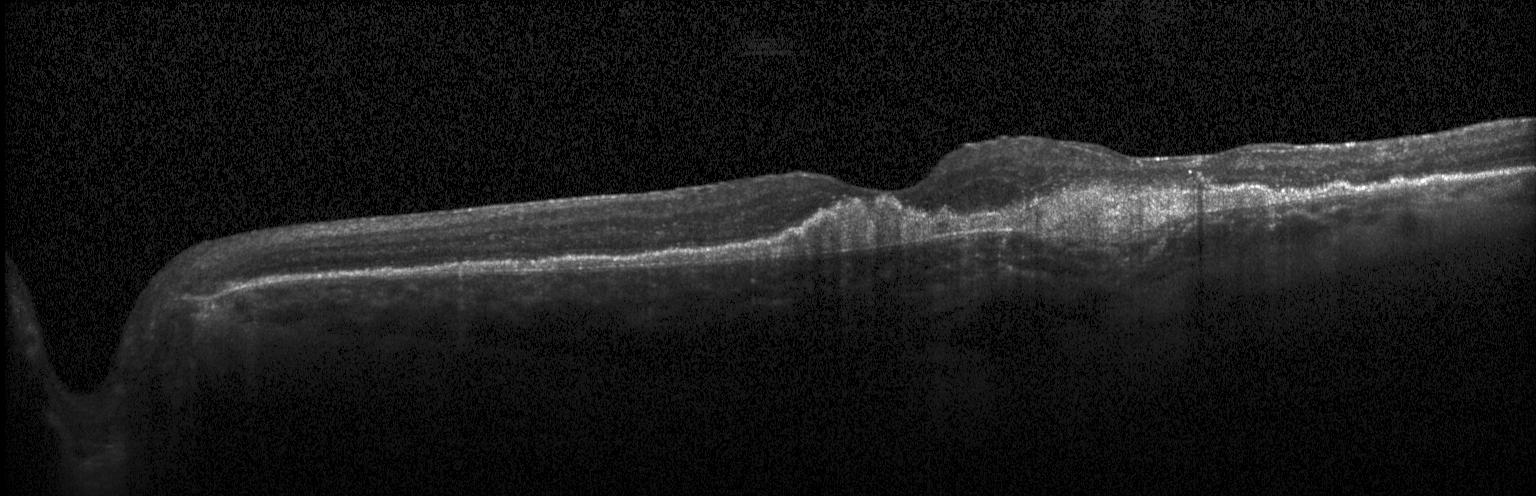 Optical coherence tomography scan — OCT finding: CNV.